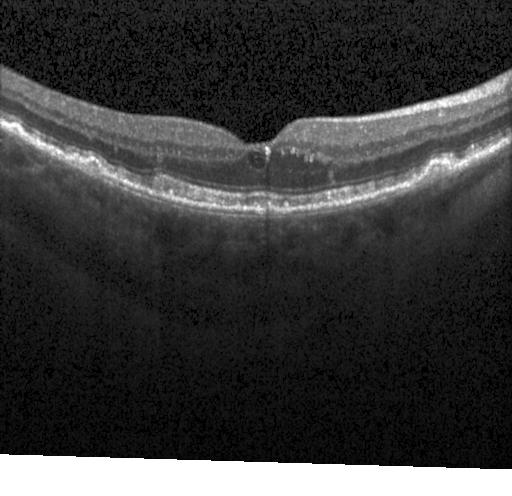
OCT B-scan, acquired on a Heidelberg Spectralis, spectral-domain optical coherence tomography
OCT finding: CNV.